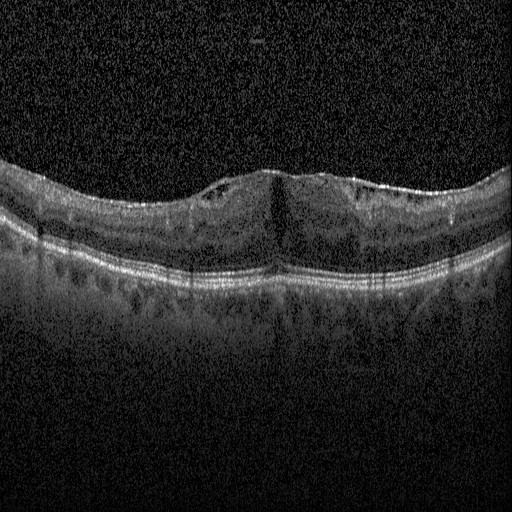 Horizontal scan through the fovea; OCT line scan; Heidelberg Spectralis OCT system — The scan shows DME.